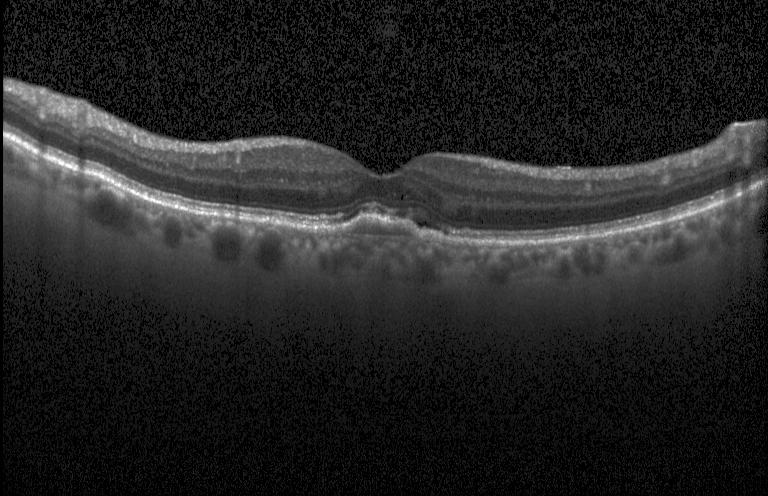
SD-OCT · OCT line scan · acquired on a Heidelberg Spectralis · horizontal scan through the fovea. The scan shows choroidal neovascularization (CNV).